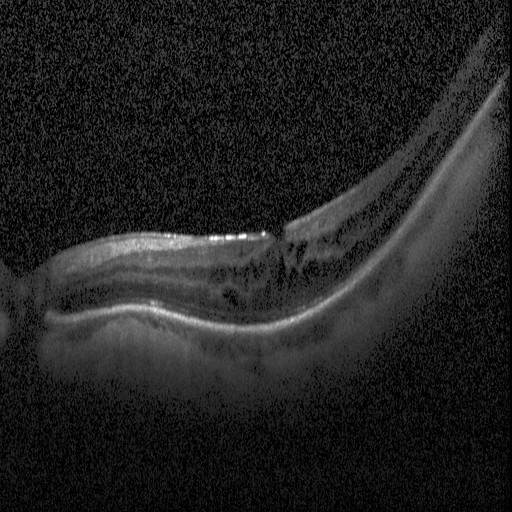

Spectral-domain optical coherence tomography, retinal OCT B-scan — Diagnosis: DME.